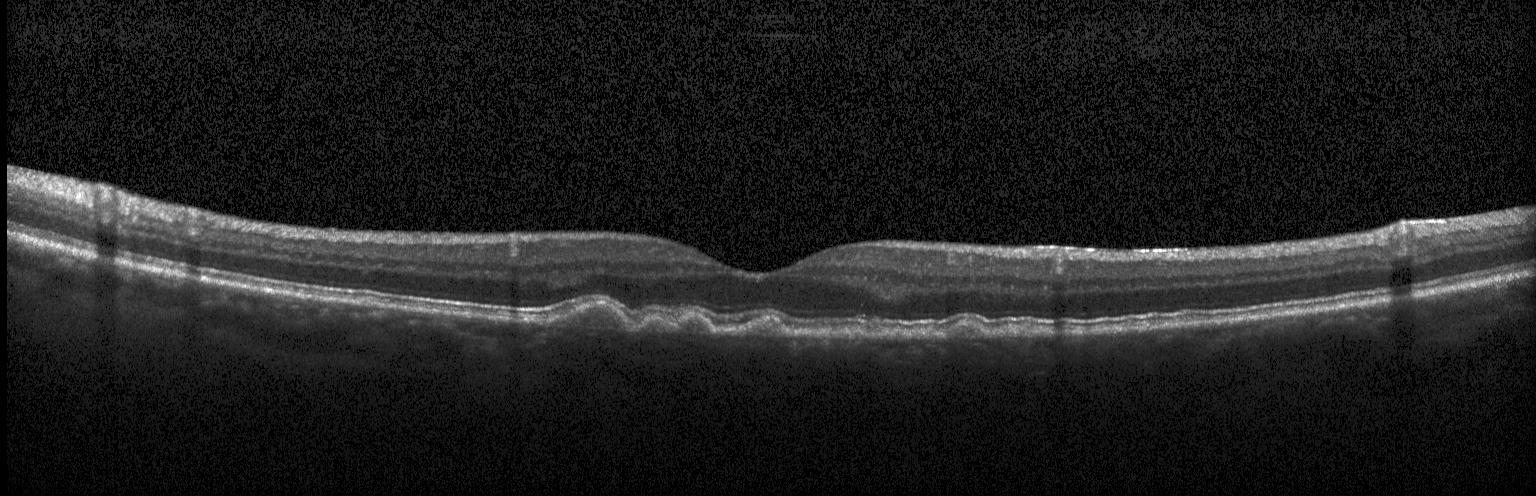
Instrument: Heidelberg Spectralis · spectral-domain optical coherence tomography · retinal OCT cross-section · fovea-centered.
Impression: multiple drusen.